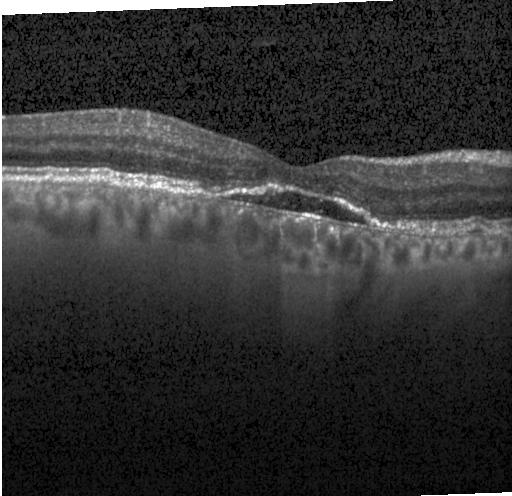 Retinal OCT cross-section · Heidelberg Spectralis OCT system · SD-OCT — A choroidal neovascular membrane.